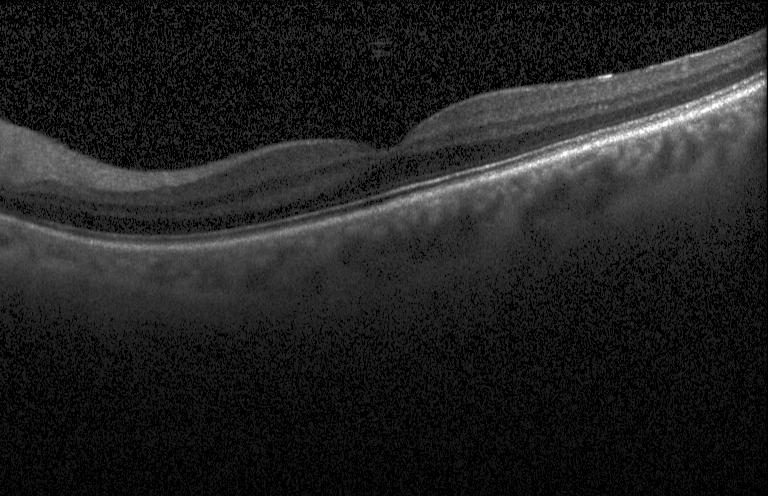 Impression: no evidence of choroidal neovascularization, diabetic macular edema, or drusen.